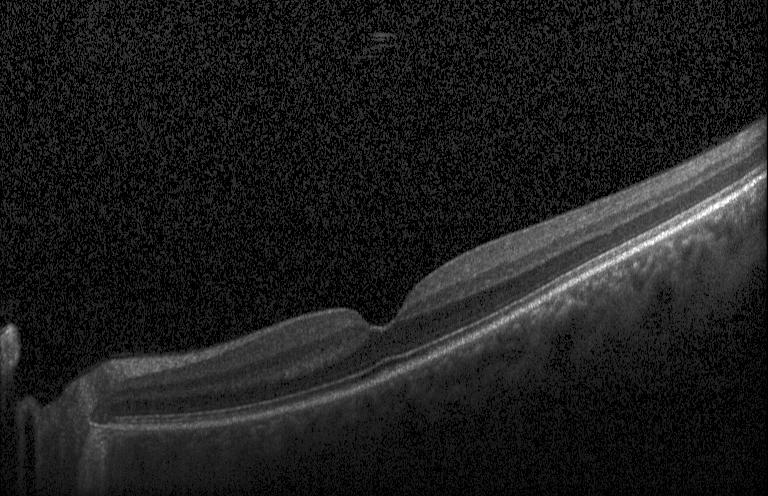

Heidelberg Spectralis · through the macula · optical coherence tomography scan · SD-OCT.
This B-scan demonstrates no choroidal neovascularization, diabetic macular edema, or drusen.